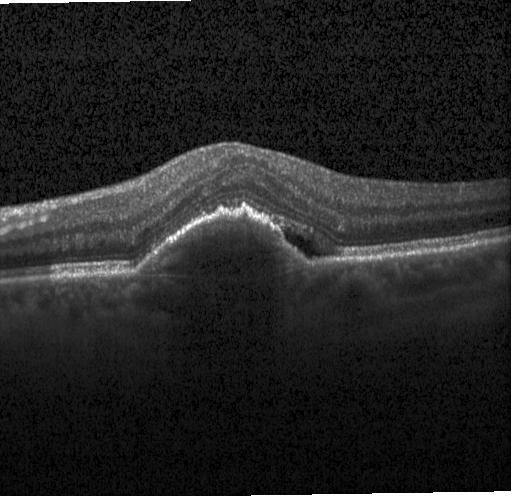
OCT B-scan
Diagnosis: a choroidal neovascular membrane.